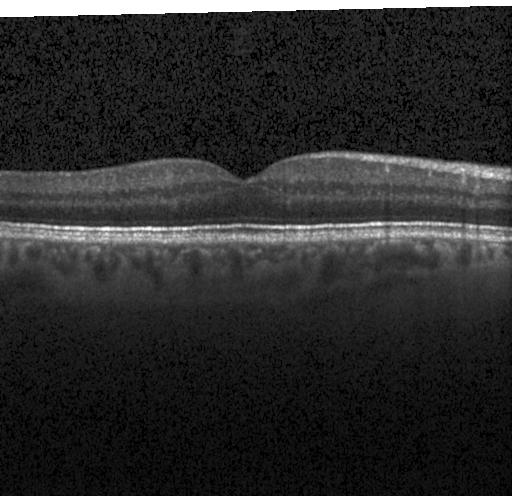

Fovea-centered; retinal OCT B-scan; SD-OCT.
Finding: neither CNV, DME, nor drusen.